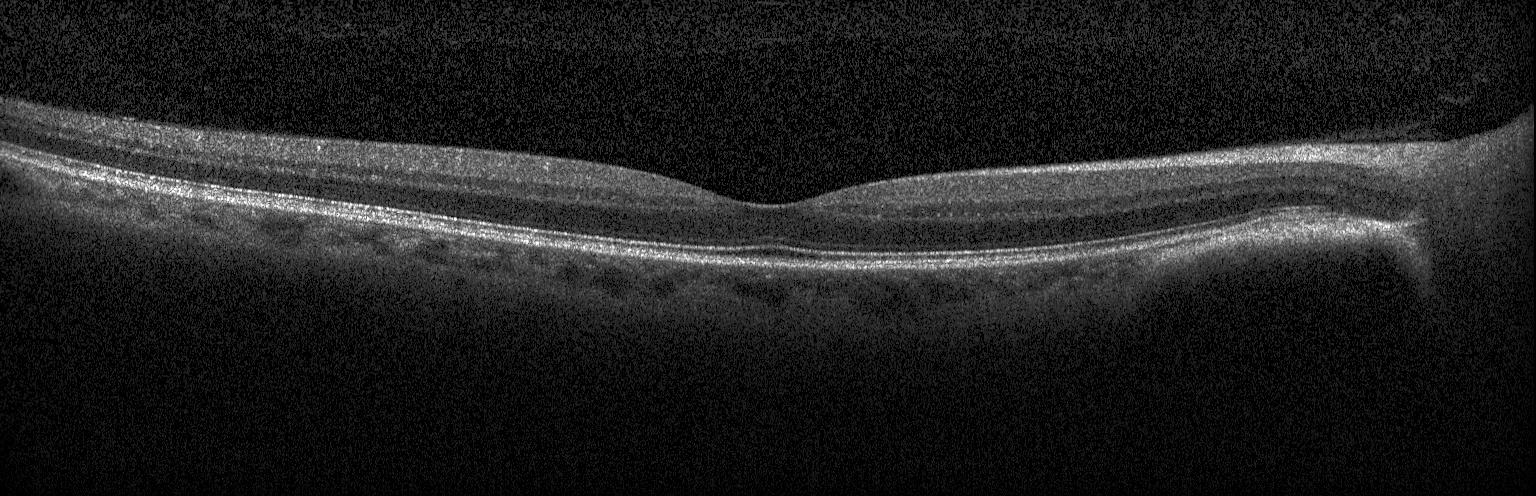 Optical coherence tomography B-scan · spectral-domain OCT · Heidelberg Spectralis — Diagnosis: no CNV, DME, or drusen.